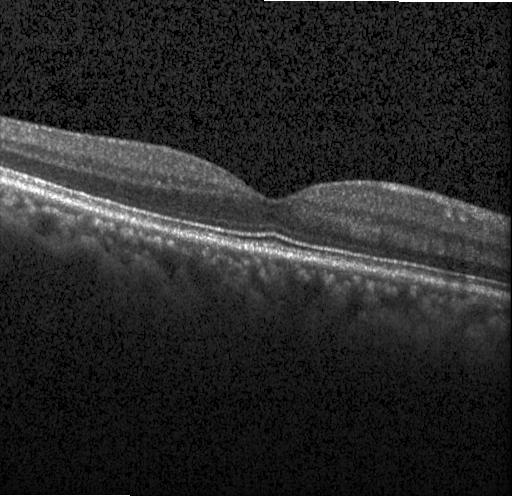
Macular scan. OCT line scan.
No CNV, DME, or drusen.